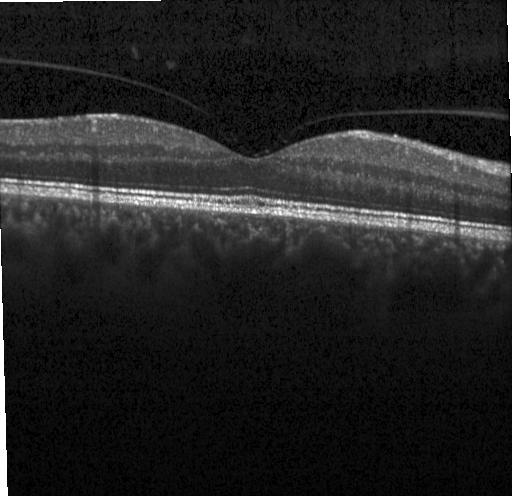 This B-scan demonstrates no evidence of choroidal neovascularization, diabetic macular edema, or drusen.